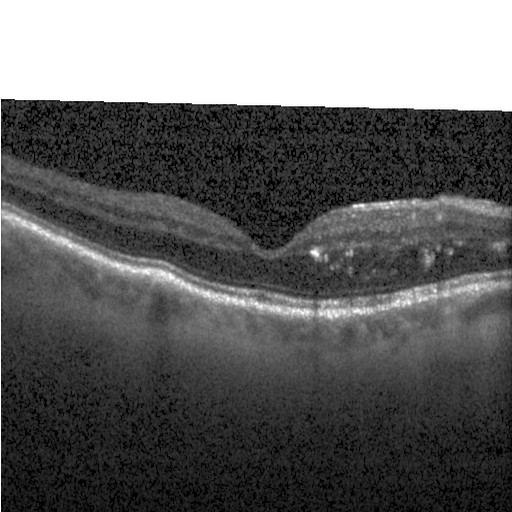
OCT line scan
OCT finding: diabetic macular edema.